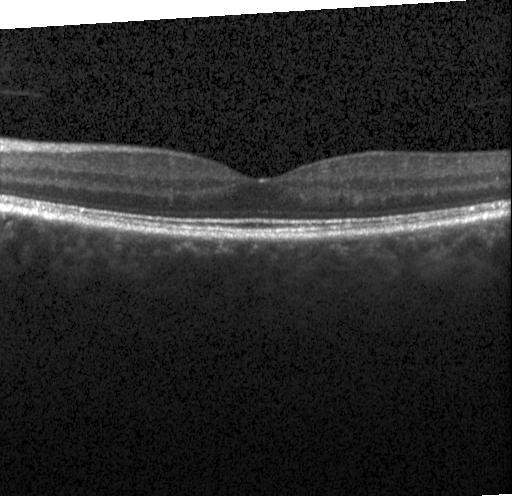 Macular OCT: neither choroidal neovascularization, diabetic macular edema, nor drusen.